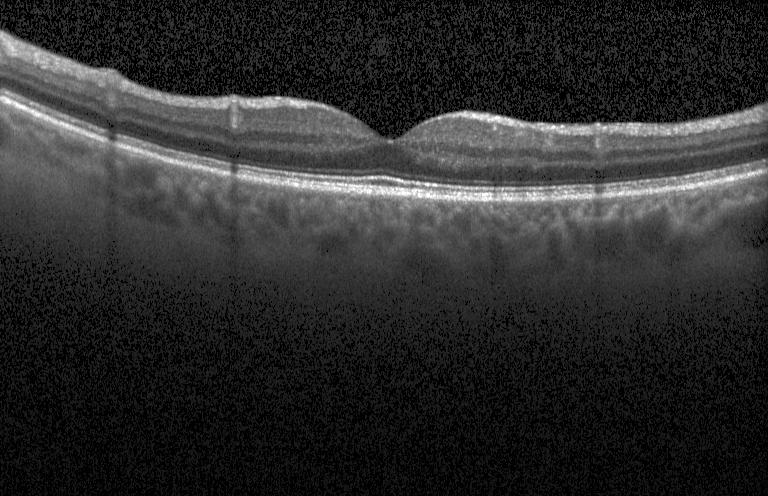

SD-OCT · optical coherence tomography B-scan · instrument: Heidelberg Spectralis · centered on the fovea
The scan shows no choroidal neovascularization, diabetic macular edema, or drusen.